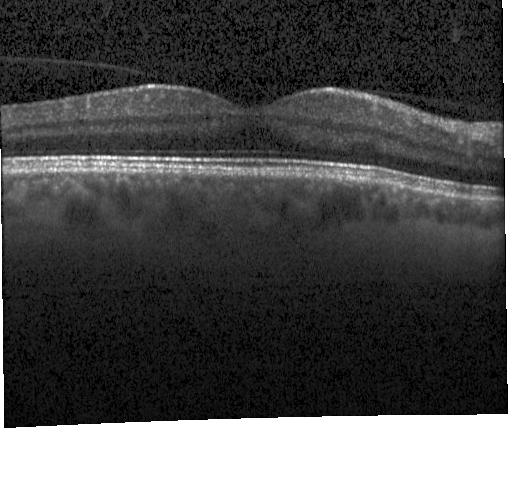
OCT B-scan. Heidelberg Spectralis OCT system. This B-scan demonstrates neither choroidal neovascularization, diabetic macular edema, nor drusen.